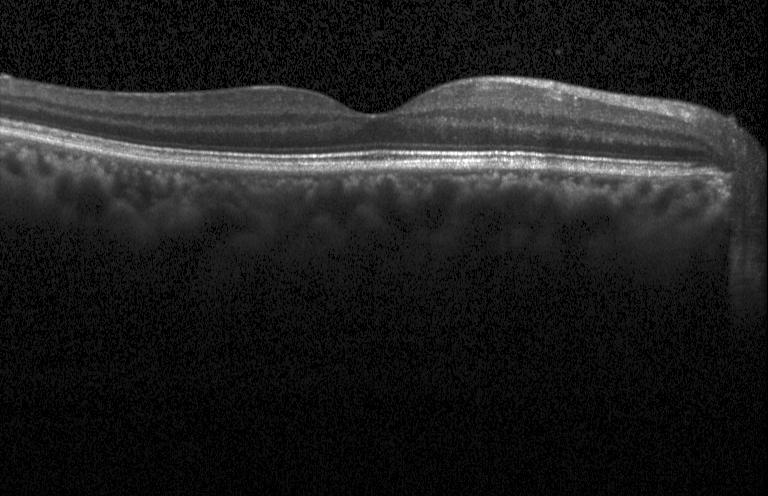 Heidelberg Spectralis OCT system · OCT B-scan.
Macular OCT: neither choroidal neovascularization, diabetic macular edema, nor drusen.